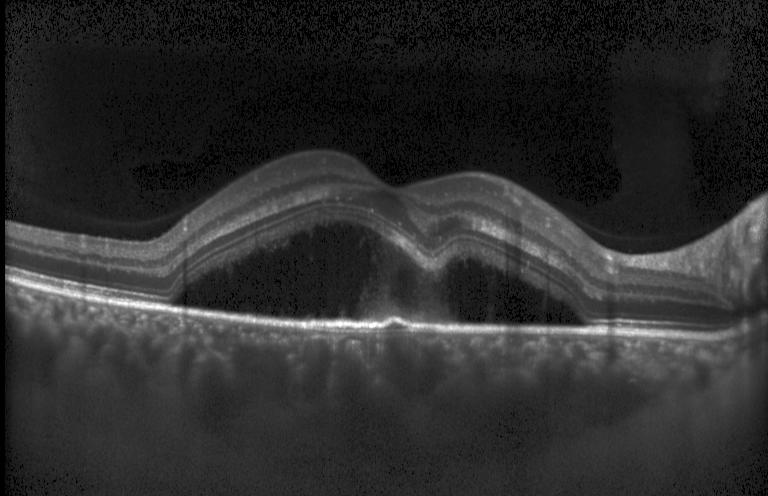
Macular OCT demonstrating a choroidal neovascular membrane.